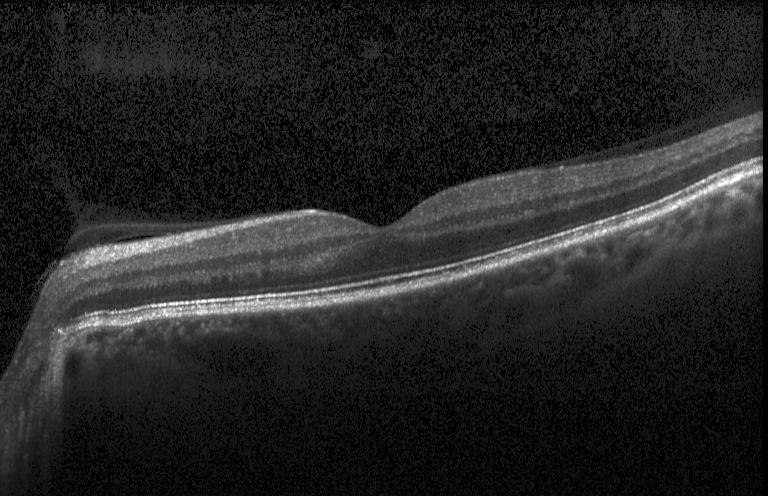
Optical coherence tomography B-scan.
The scan shows no choroidal neovascularization, no diabetic macular edema, and no drusen.